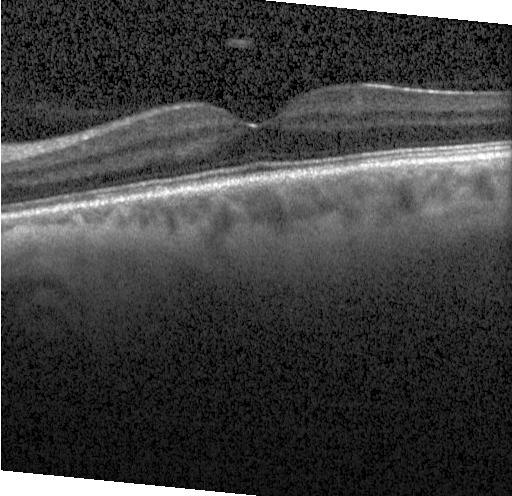

Spectral-domain optical coherence tomography · OCT B-scan · Heidelberg Spectralis OCT system
Diagnosis: no evidence of CNV, DME, or drusen.